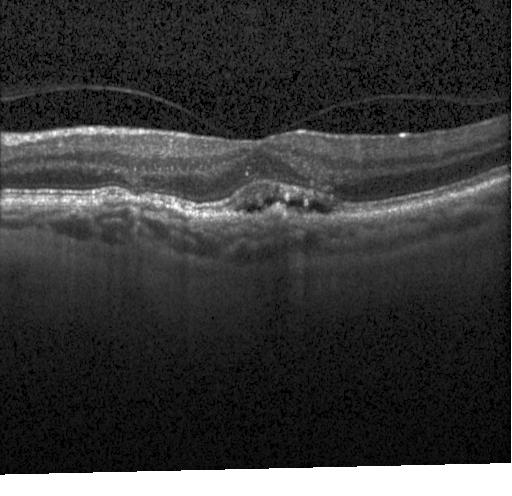 The scan shows a choroidal neovascular membrane.